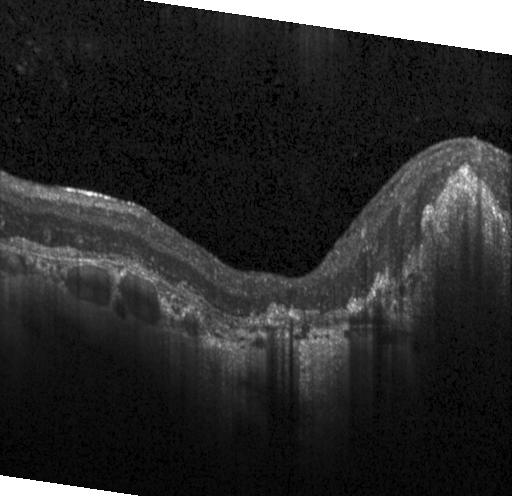 Spectral-domain OCT B-scan: a choroidal neovascular membrane.